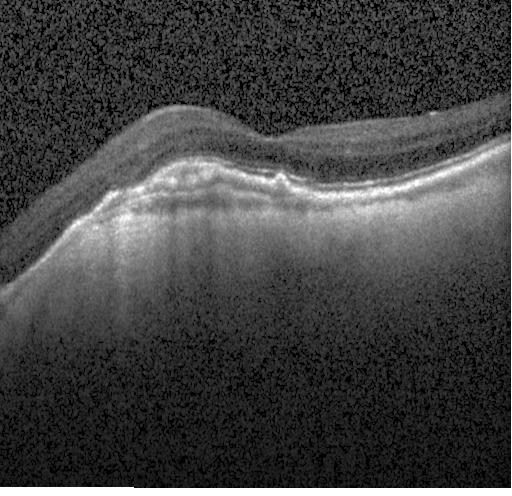 Fovea-centered · optical coherence tomography B-scan
Diagnosis: a choroidal neovascular membrane.